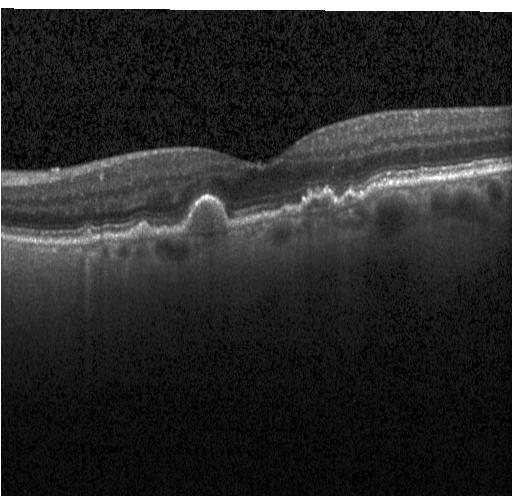 OCT B-scan. Diagnosis: drusen.